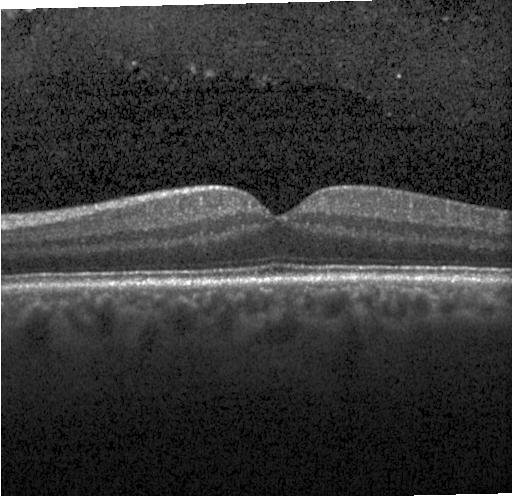
Spectral-domain optical coherence tomography · Heidelberg Spectralis · OCT line scan
Macular OCT: no choroidal neovascularization, diabetic macular edema, or drusen.